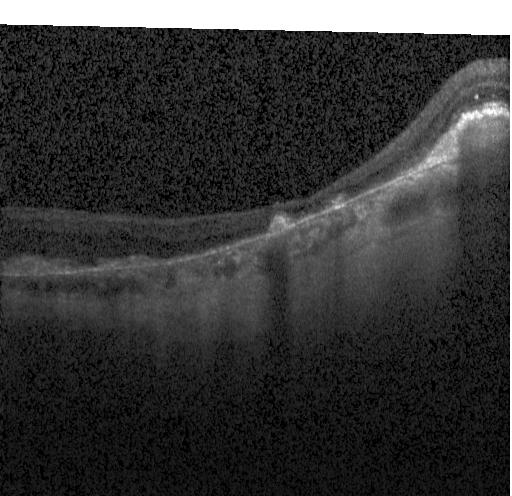

Macular OCT: choroidal neovascularization (CNV).